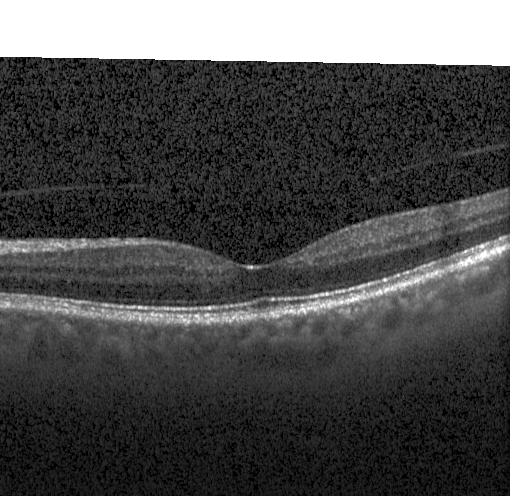
Spectral-domain optical coherence tomography. Optical coherence tomography B-scan.
Impression: no evidence of choroidal neovascularization, diabetic macular edema, or drusen.